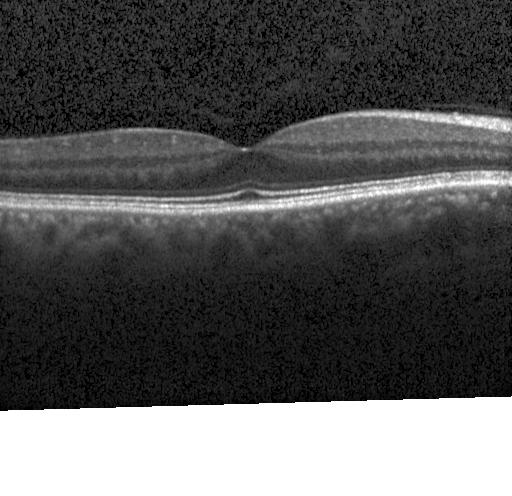 OCT B-scan · spectral-domain OCT — Finding: neither CNV, DME, nor drusen.